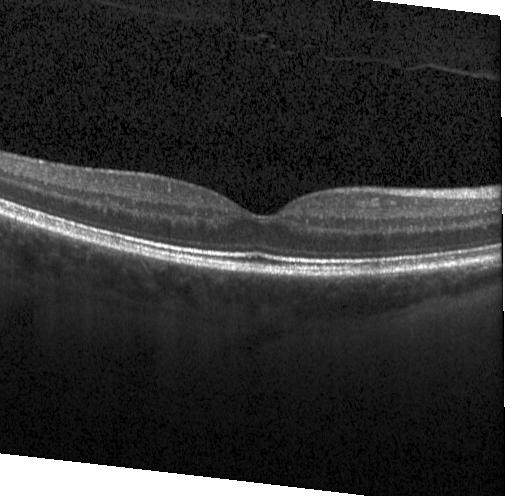

Impression: no choroidal neovascularization, no diabetic macular edema, and no drusen.